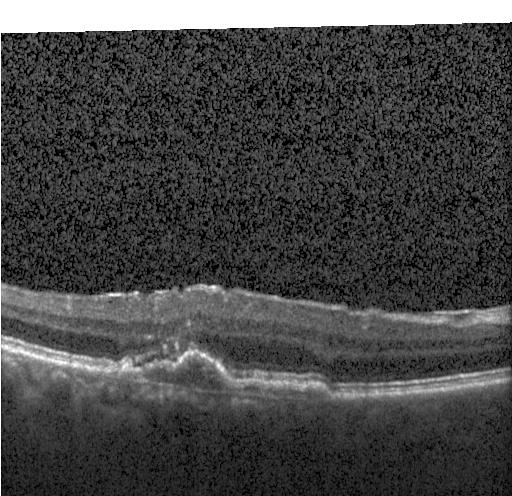 Macular OCT: a choroidal neovascular membrane.